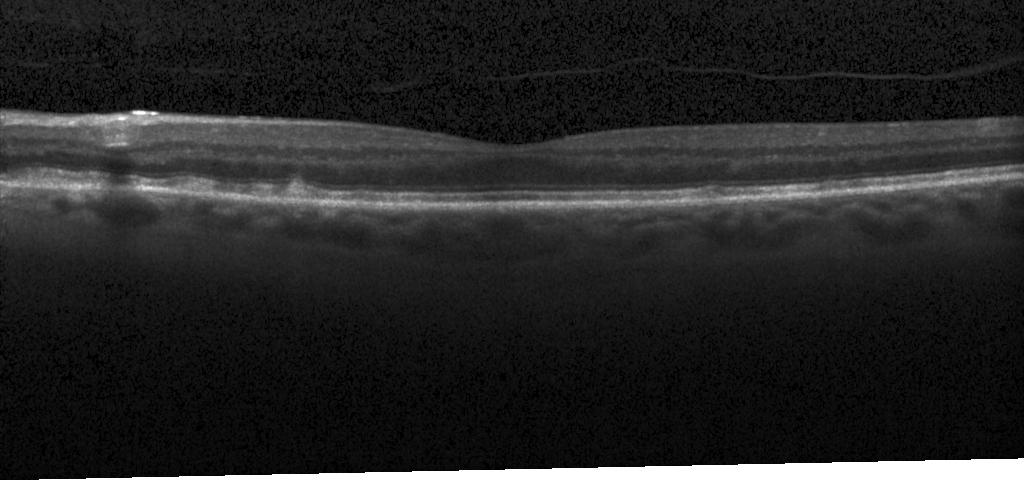

Retinal OCT cross-section · spectral-domain OCT
Impression: sub-RPE drusenoid deposits.